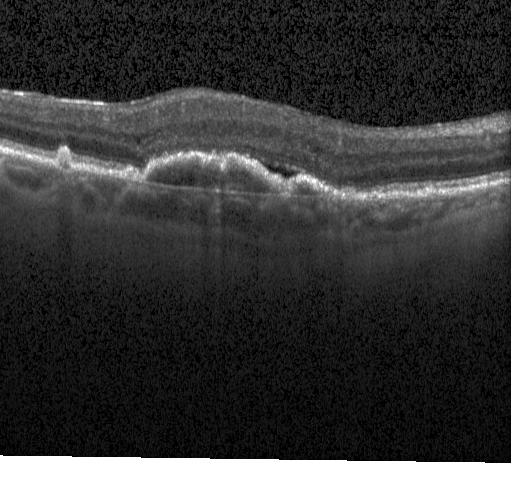

OCT scan showing choroidal neovascularization (CNV).